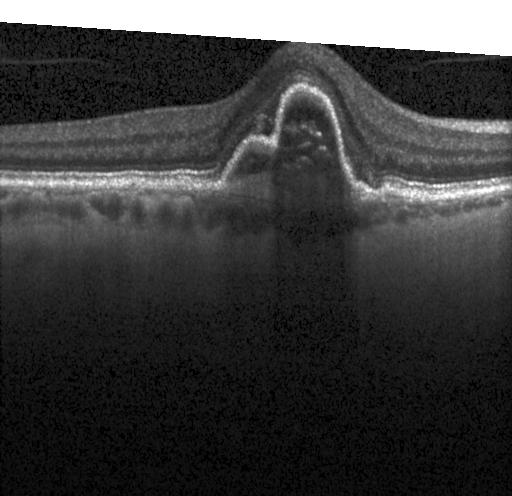 Choroidal neovascularization.